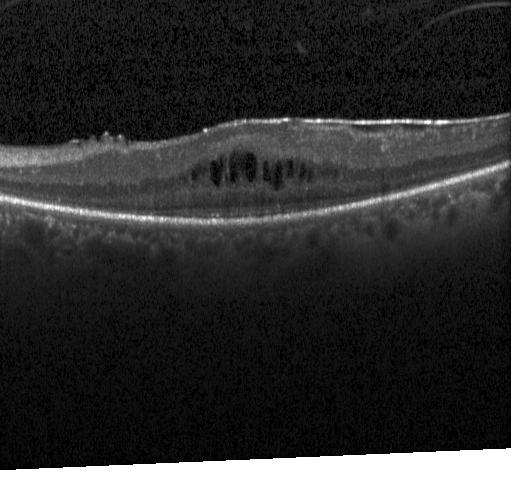
Retinal OCT B-scan
Diagnosis: diabetic macular edema (DME).